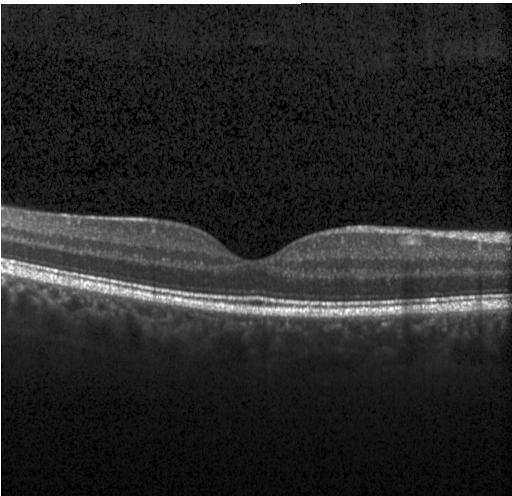

No evidence of CNV, DME, or drusen.